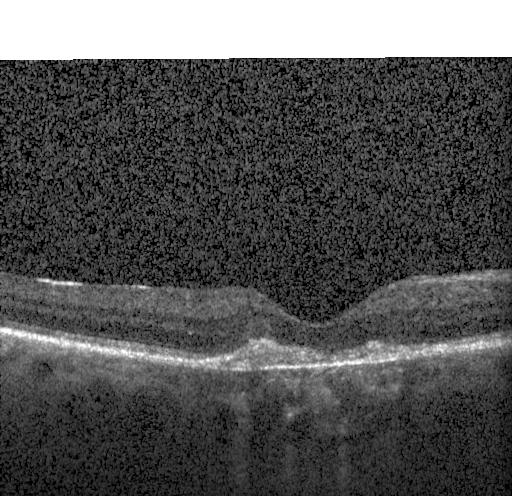
SD-OCT; OCT line scan
This B-scan demonstrates a choroidal neovascular membrane.